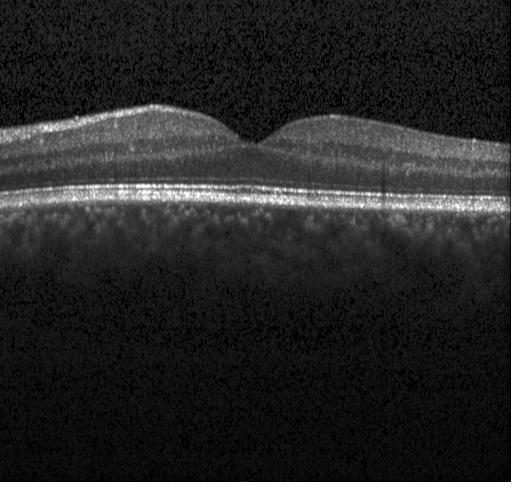 Diagnosis: no choroidal neovascularization, diabetic macular edema, or drusen.